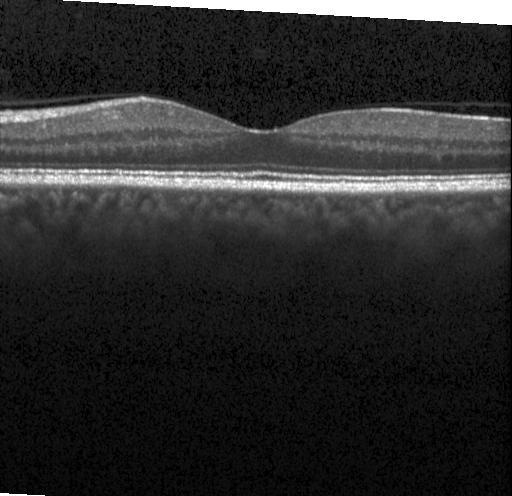
Finding: no CNV, no DME, and no drusen.